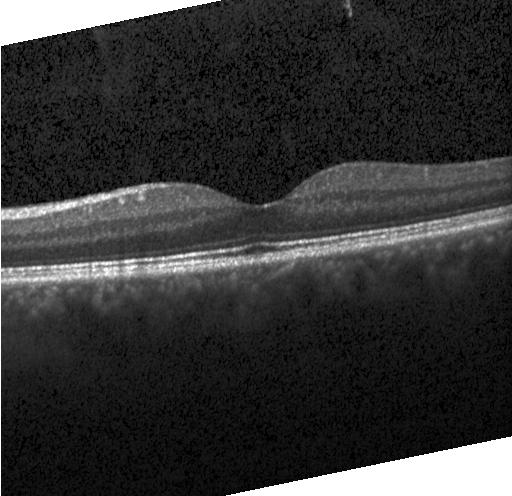

Assessment: no choroidal neovascularization, no diabetic macular edema, and no drusen.